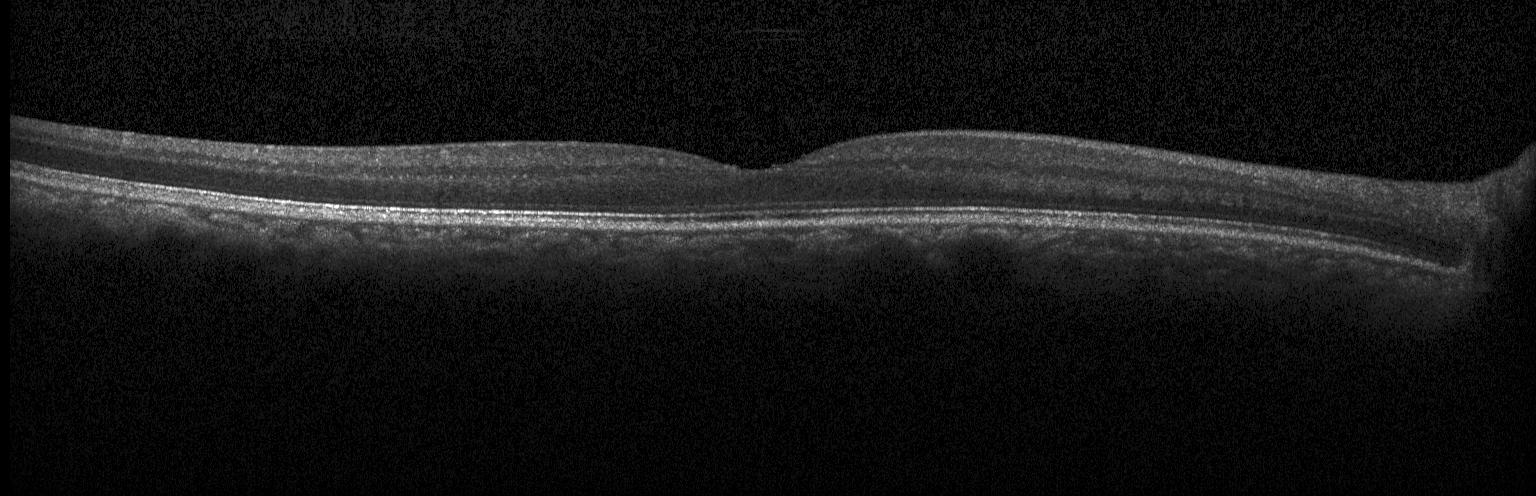 Heidelberg Spectralis OCT system. Horizontal scan through the fovea. Retinal OCT B-scan. Spectral-domain OCT — OCT finding: no choroidal neovascularization, diabetic macular edema, or drusen.